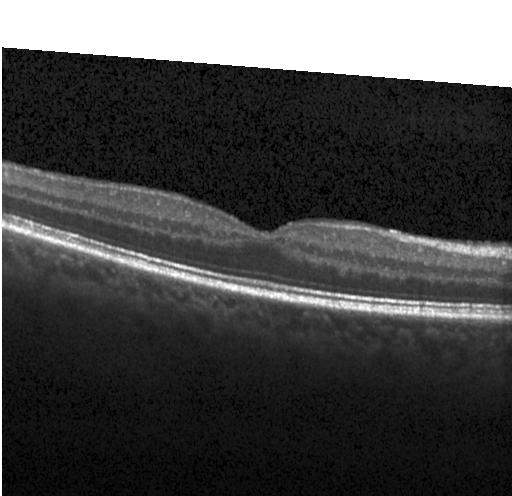
Assessment: no evidence of choroidal neovascularization, diabetic macular edema, or drusen.